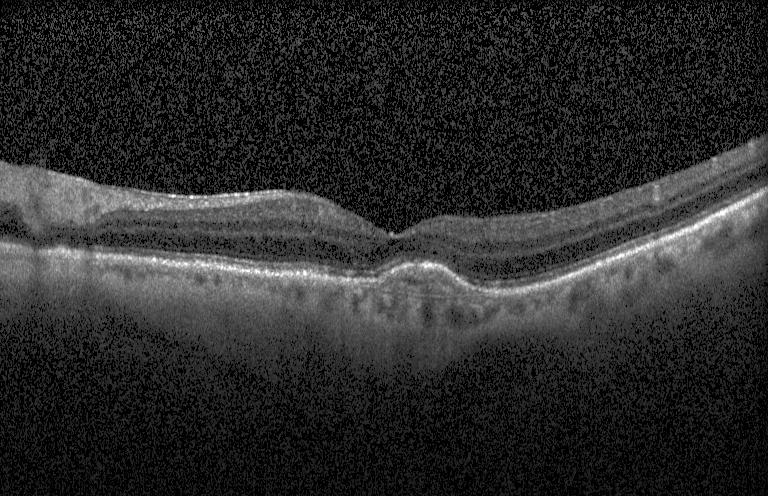 Fovea-centered. Optical coherence tomography B-scan.
Impression: a choroidal neovascular membrane.